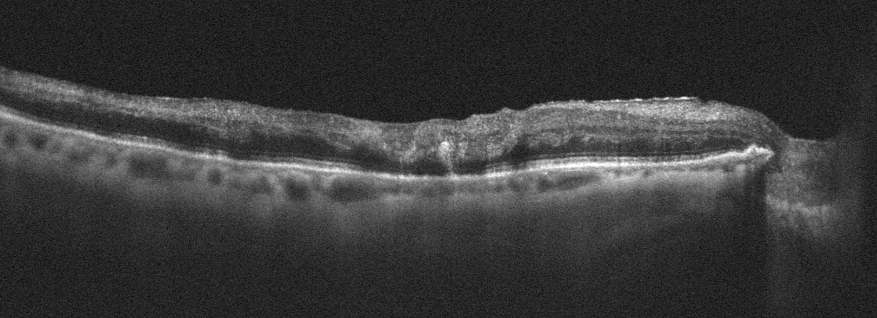

Retinal OCT cross-section
Diagnosis: diabetic macular edema.